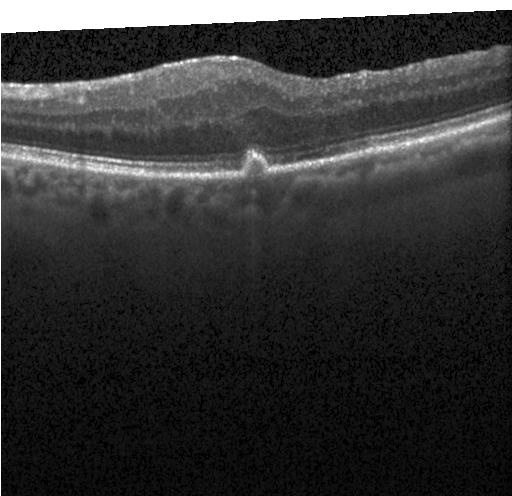

OCT B-scan — Finding: sub-RPE drusenoid deposits.